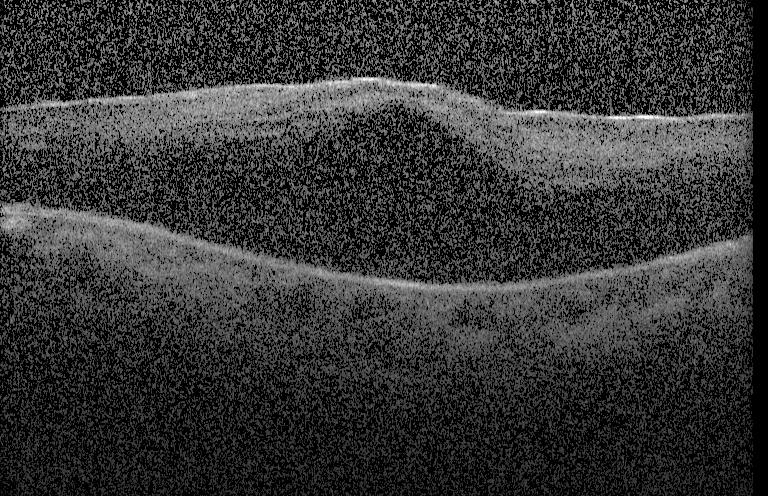

OCT B-scan. Diabetic macular edema.